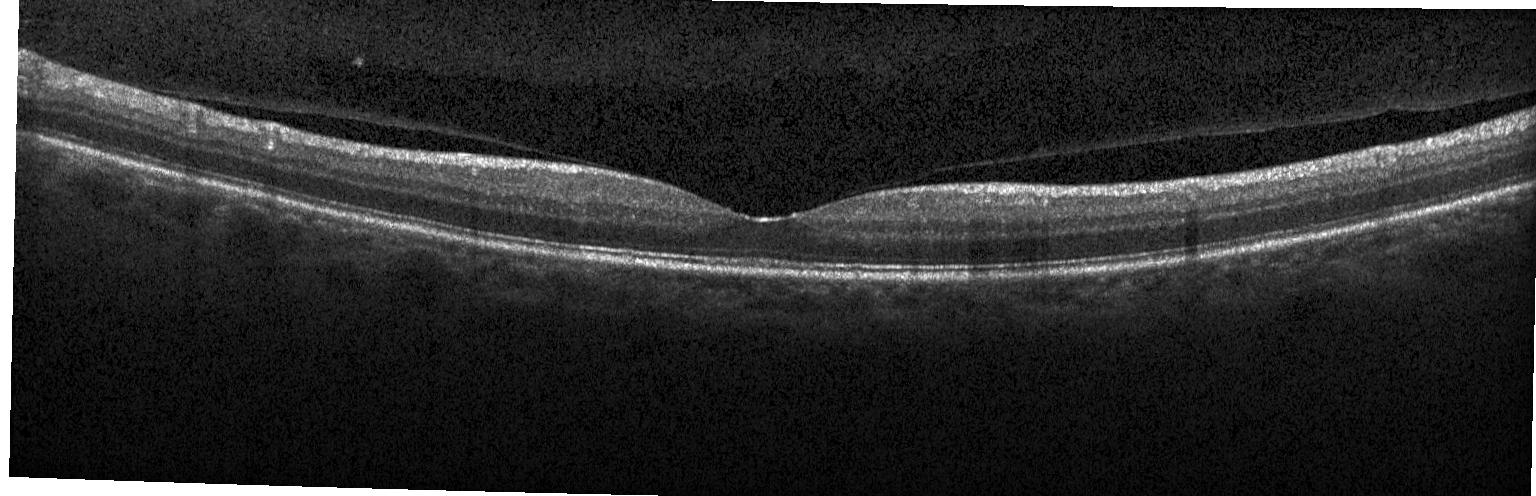 Heidelberg Spectralis OCT system; OCT B-scan
Finding: no evidence of CNV, DME, or drusen.